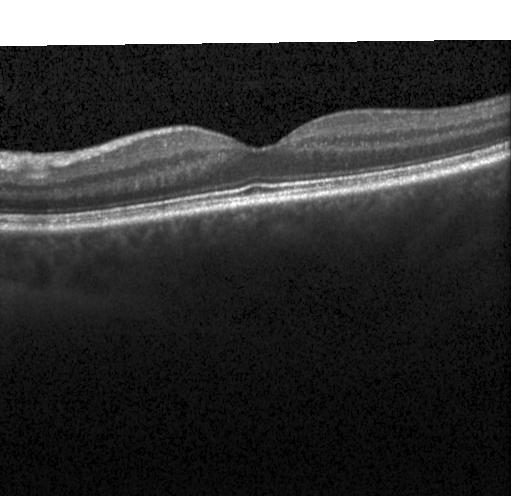
Retinal OCT B-scan · macular scan · acquired on a Heidelberg Spectralis. Impression: no CNV, DME, or drusen.